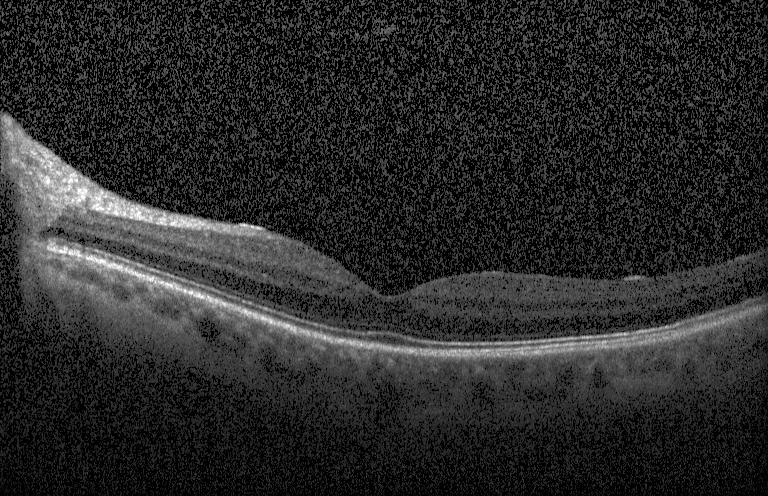

Fovea-centered · OCT line scan
Macular OCT: no evidence of choroidal neovascularization, diabetic macular edema, or drusen.